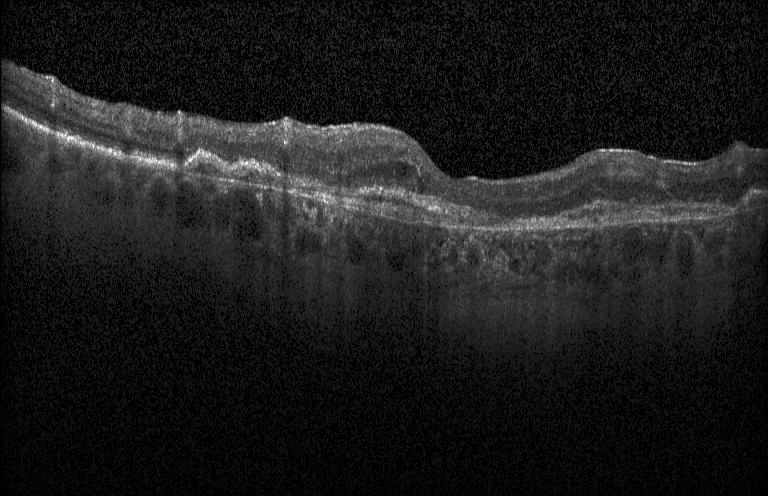
OCT line scan — Diagnosis: CNV.